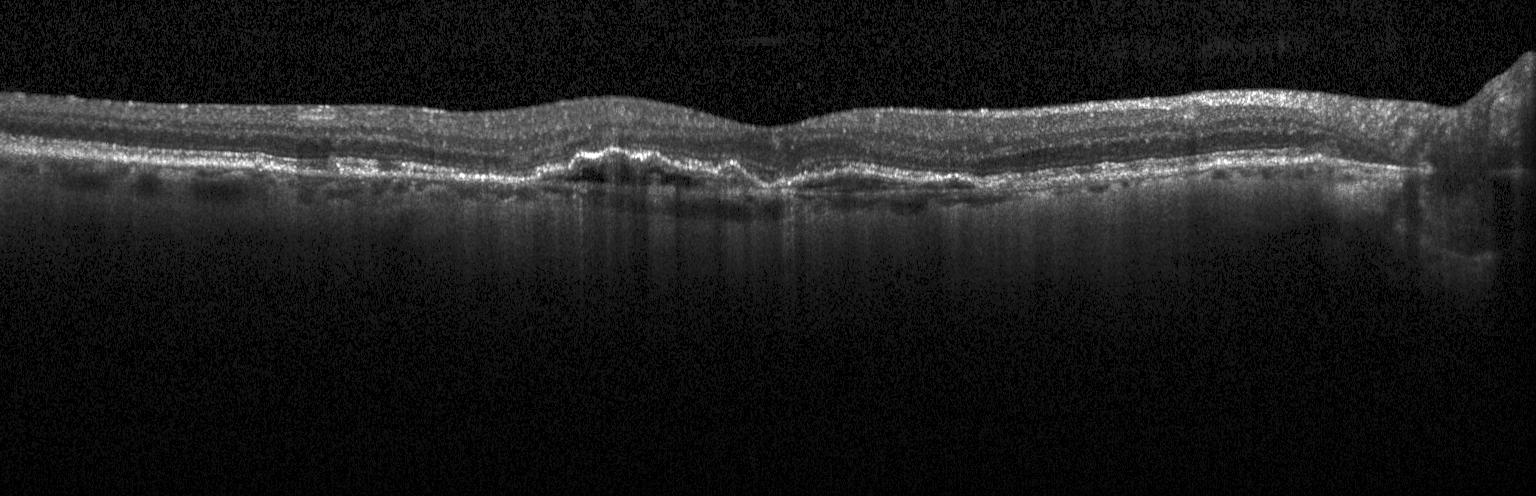
Through the macula; OCT line scan — Finding: a choroidal neovascular membrane.